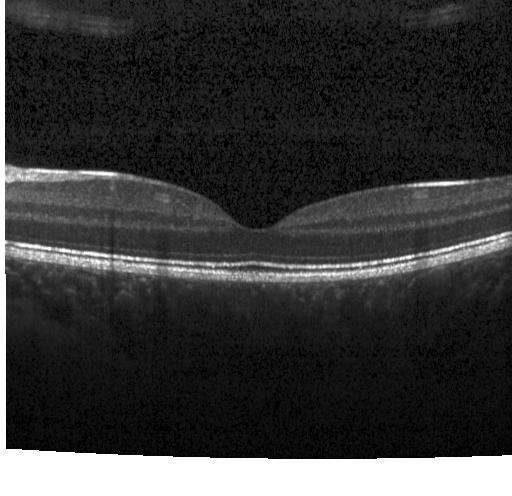 Spectral-domain OCT B-scan: no evidence of choroidal neovascularization, diabetic macular edema, or drusen.